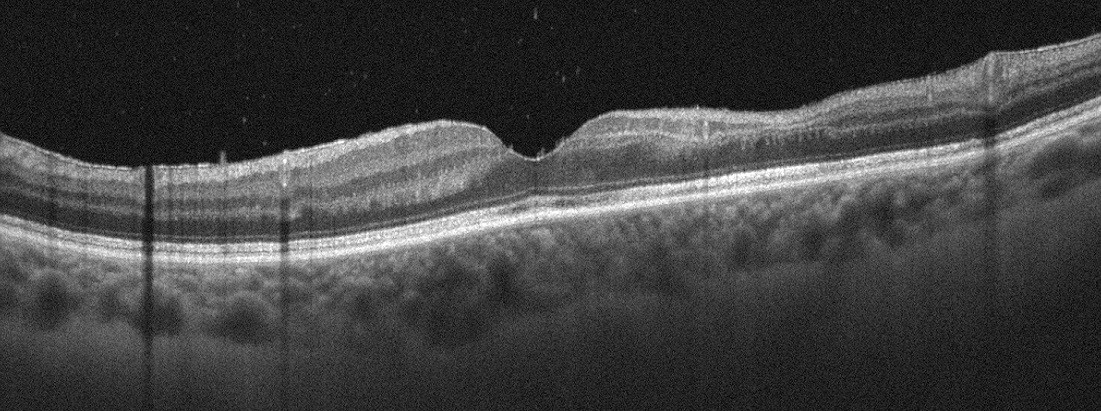 Fovea-centered · optical coherence tomography B-scan. Finding: retinal vein occlusion (RVO).